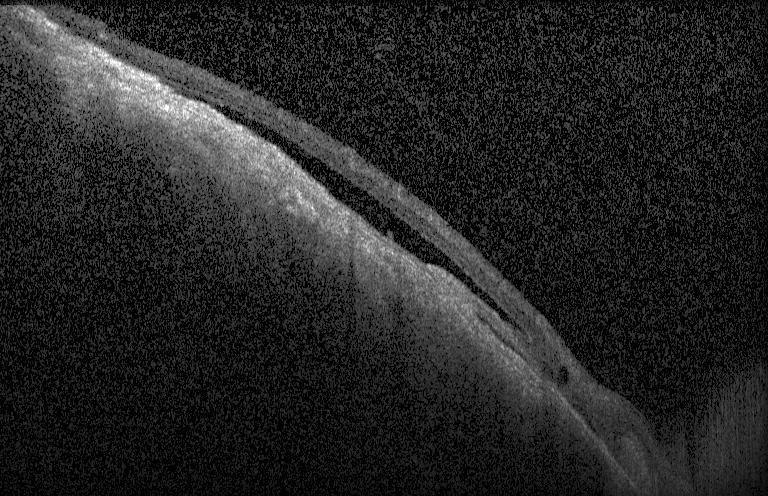 Macular OCT demonstrating a choroidal neovascular membrane.